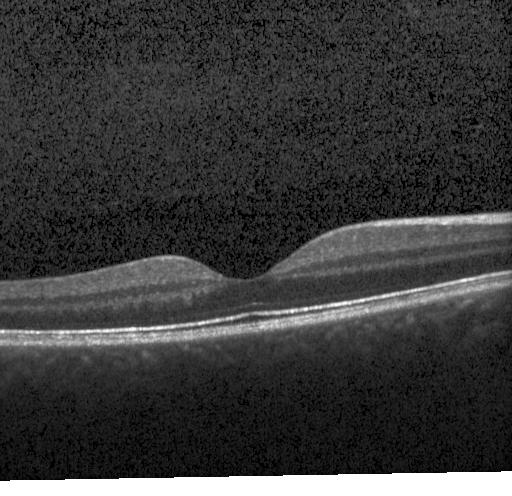

The scan shows neither CNV, DME, nor drusen.